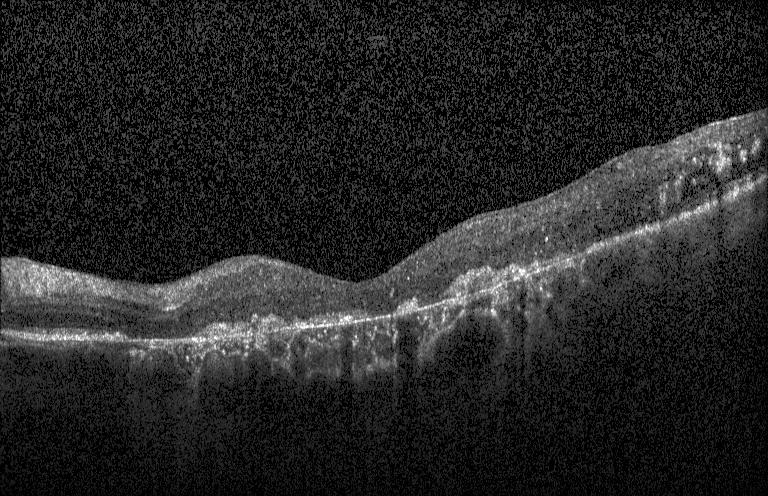

Optical coherence tomography B-scan.
Choroidal neovascularization.